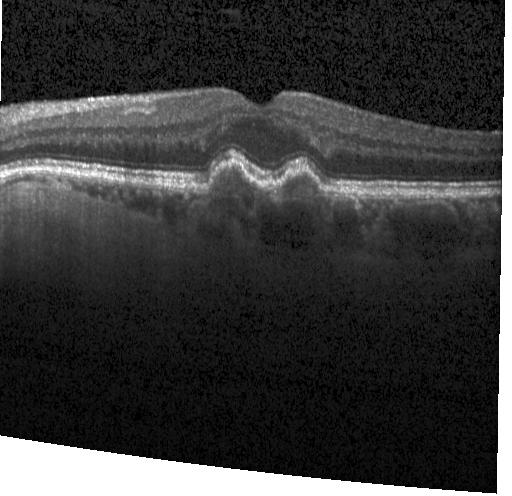
Finding: a choroidal neovascular membrane.